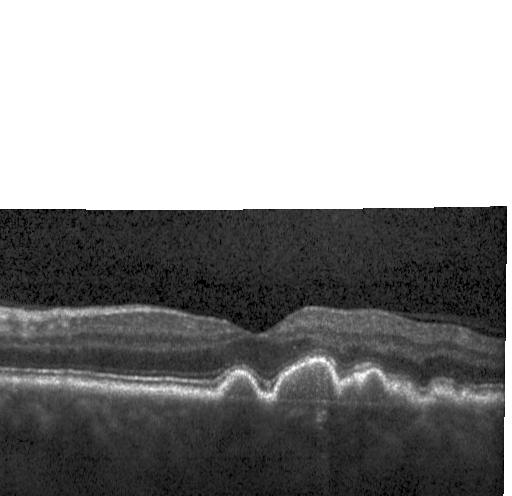
Acquired on a Heidelberg Spectralis; fovea-centered; optical coherence tomography scan; spectral-domain optical coherence tomography. Assessment: multiple drusen.